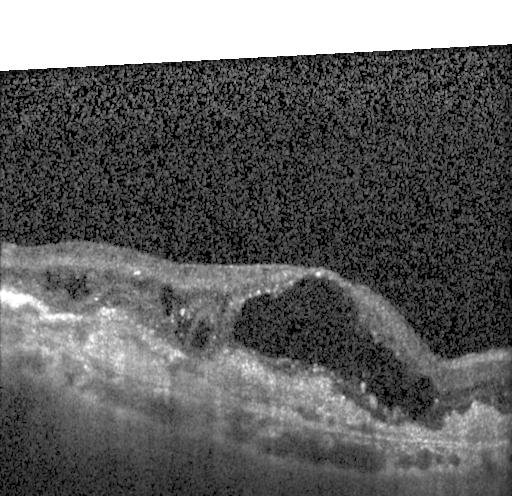 Optical coherence tomography B-scan.
Finding: choroidal neovascularization.